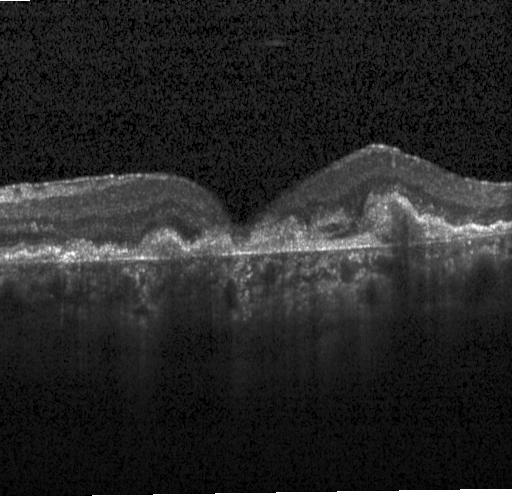 Diagnosis: a choroidal neovascular membrane.